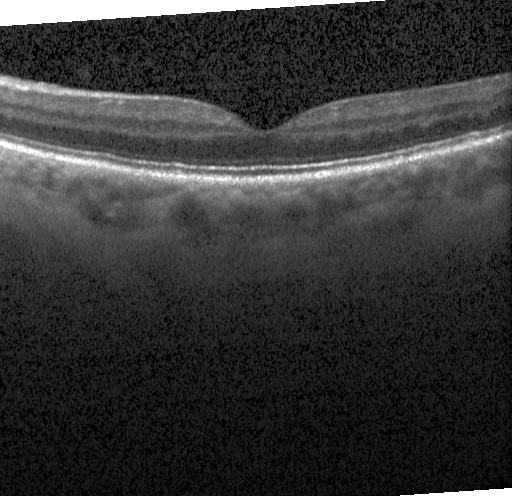

OCT line scan. Through the macula.
No choroidal neovascularization, diabetic macular edema, or drusen.